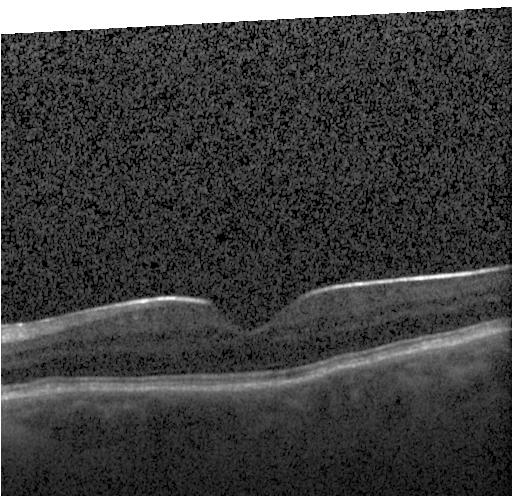 Diagnosis: no evidence of CNV, DME, or drusen.